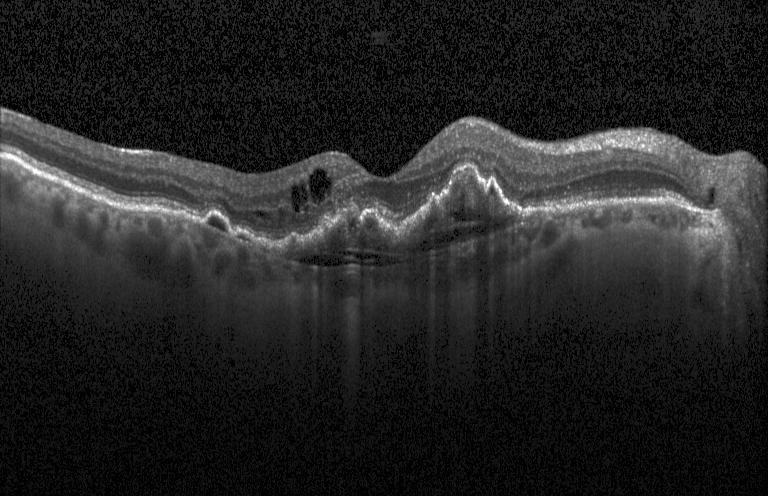

Diagnosis: choroidal neovascularization.